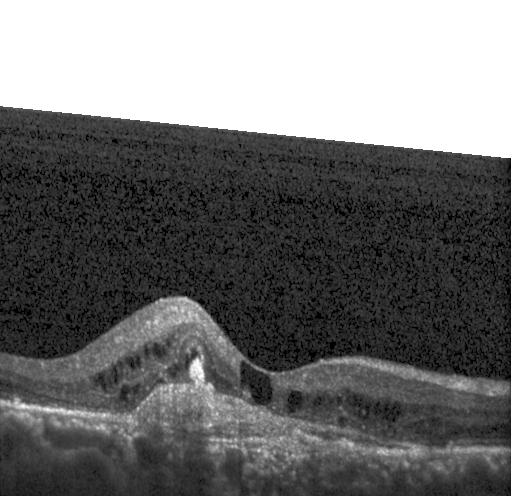

Retinal OCT cross-section; through the macula — OCT finding: a choroidal neovascular membrane.